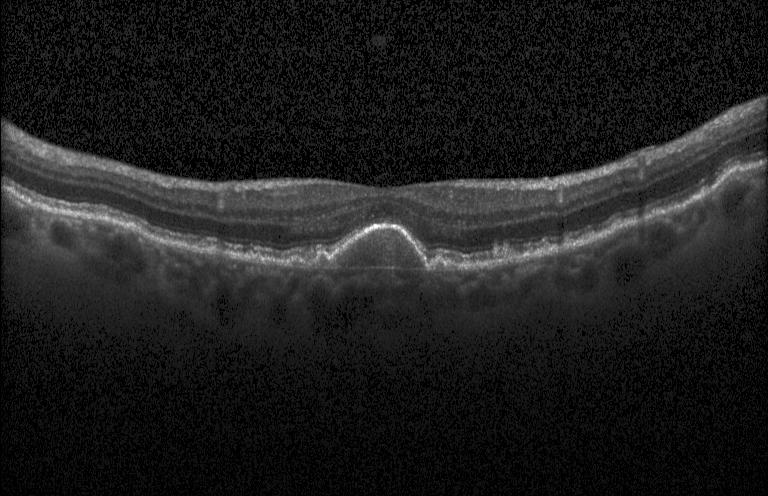

Centered on the fovea; OCT B-scan — Macular OCT: sub-RPE drusenoid deposits.